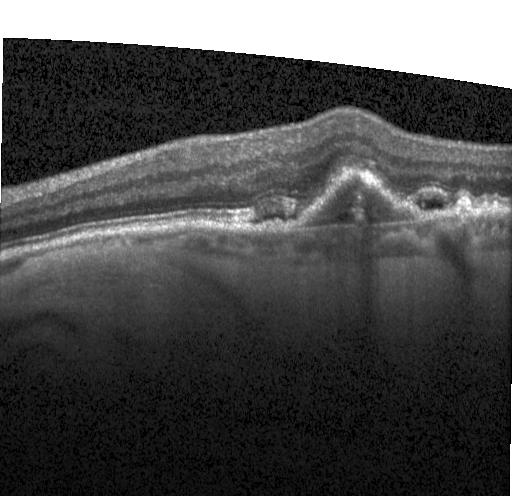

The scan shows choroidal neovascularization (CNV).